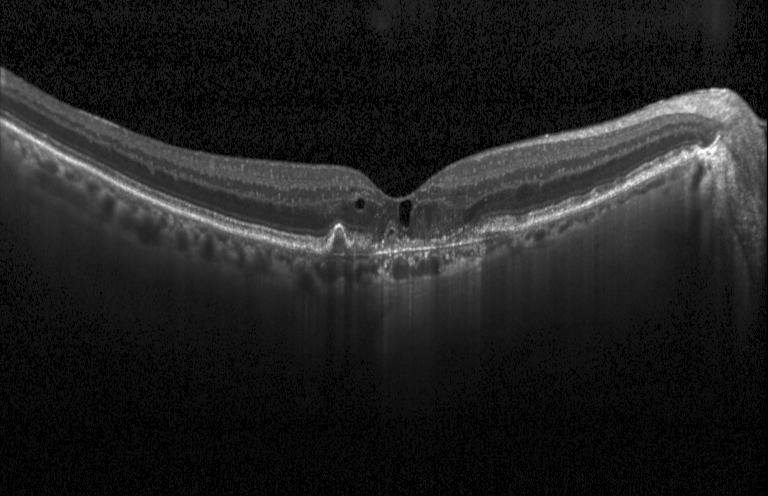
Dx: a choroidal neovascular membrane.